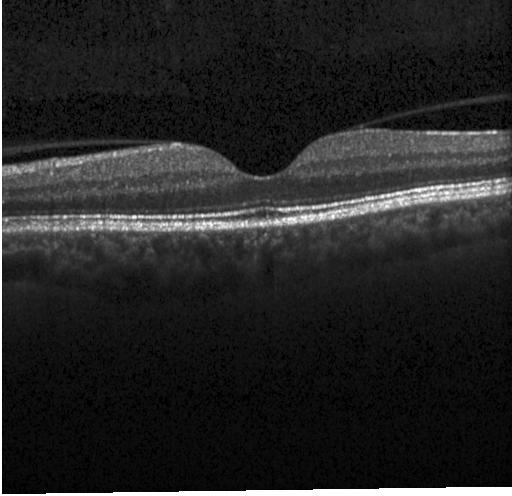 SD-OCT · instrument: Heidelberg Spectralis · macular scan · retinal OCT cross-section
This B-scan demonstrates no CNV, no DME, and no drusen.